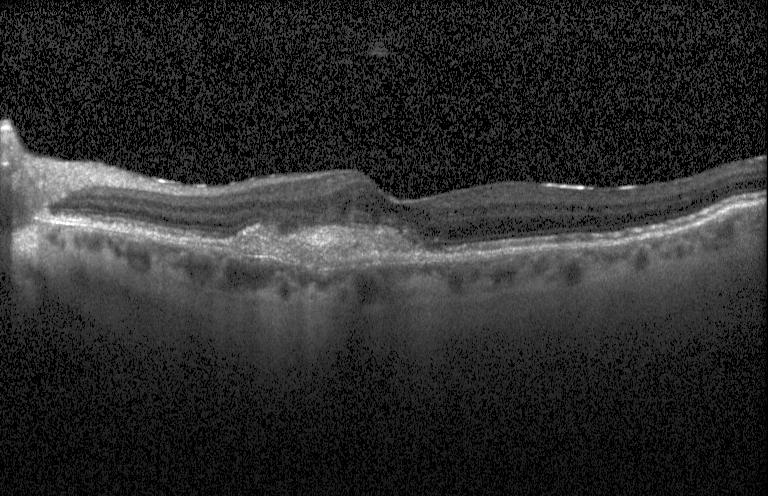 Optical coherence tomography B-scan. Finding: choroidal neovascularization.